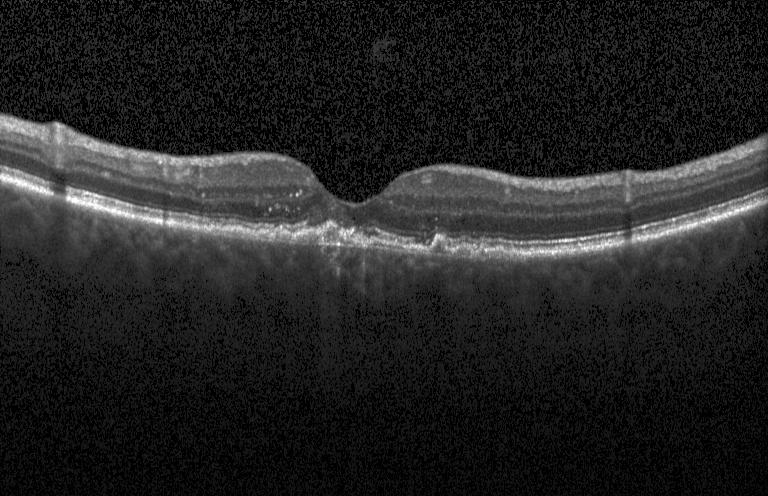

Optical coherence tomography B-scan. Through the macula. Acquired on a Heidelberg Spectralis. Spectral-domain optical coherence tomography
Assessment: a choroidal neovascular membrane.